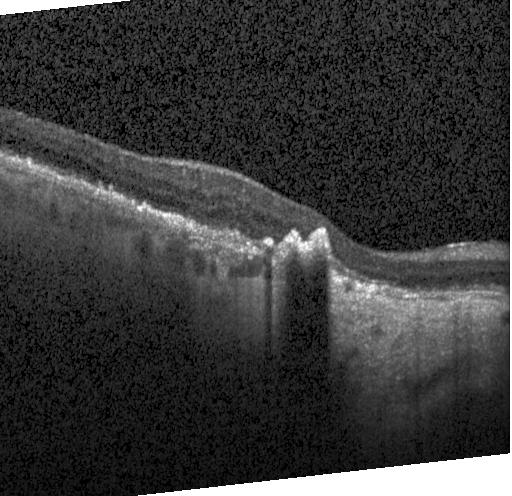

Spectral-domain optical coherence tomography. OCT line scan — Impression: a choroidal neovascular membrane.